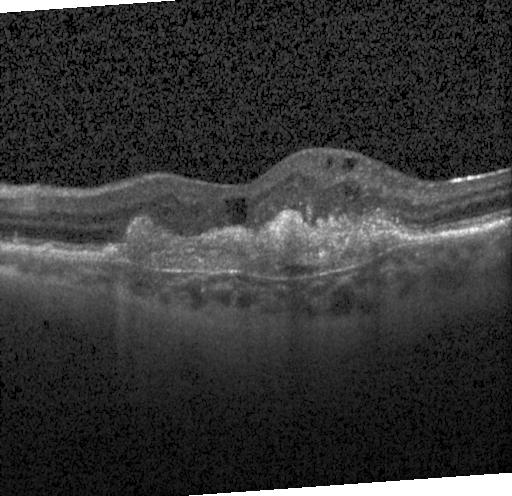

Retinal OCT B-scan; acquired on a Heidelberg Spectralis; spectral-domain optical coherence tomography; centered on the fovea — Finding: a choroidal neovascular membrane.